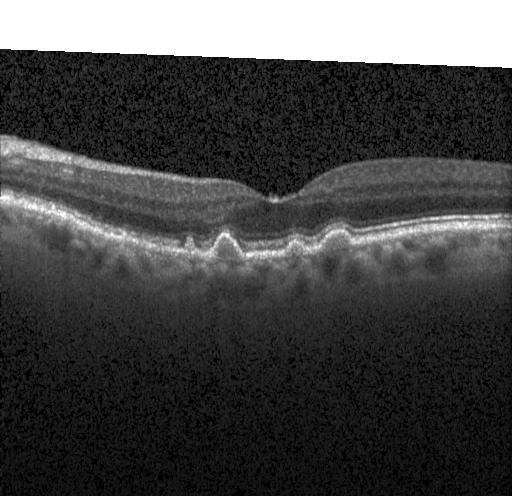
Acquired on a Heidelberg Spectralis · optical coherence tomography scan · spectral-domain optical coherence tomography — Finding: multiple drusen.